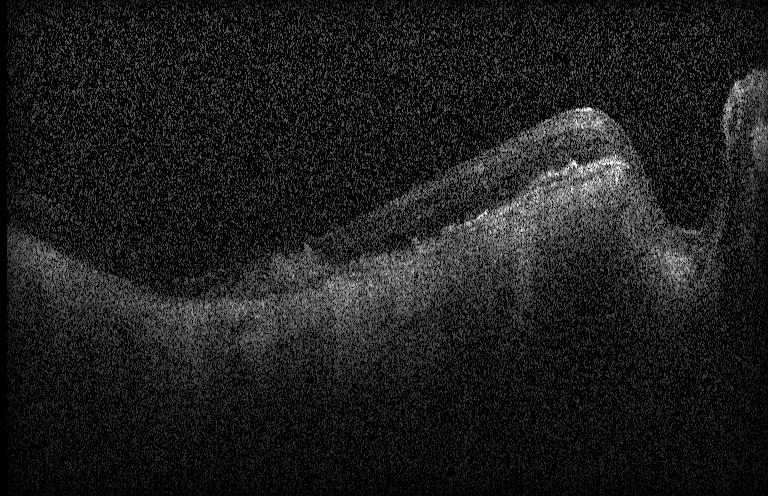

Diagnosis: a choroidal neovascular membrane.